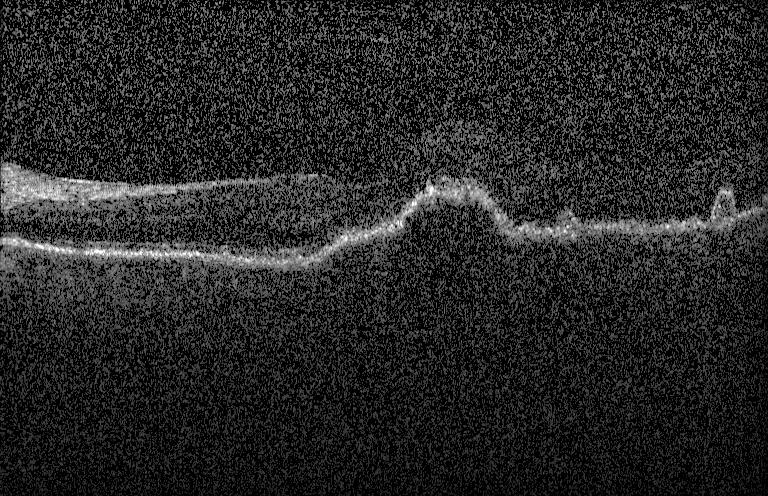
Retinal OCT cross-section — Diagnosis: choroidal neovascularization.